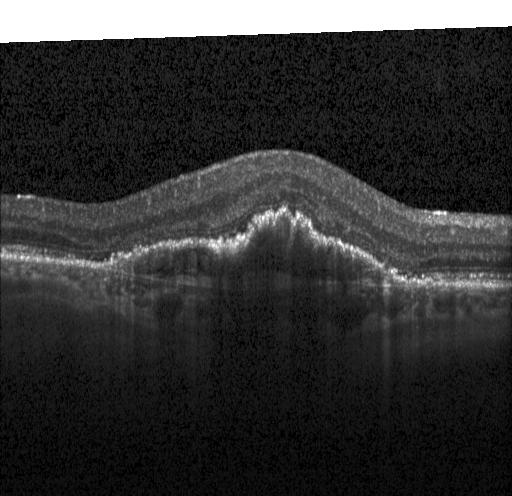 Macular OCT: a choroidal neovascular membrane.